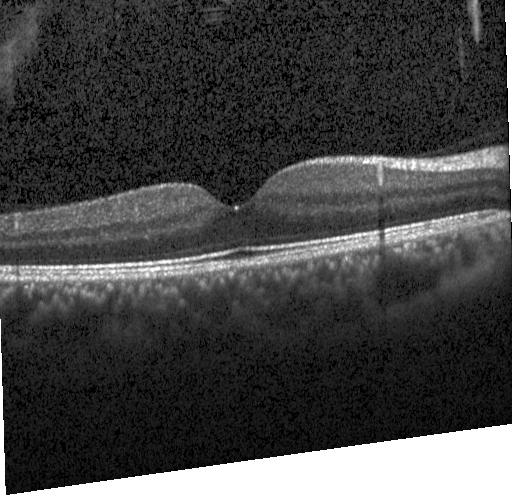

Optical coherence tomography B-scan. Heidelberg Spectralis. Fovea-centered. Spectral-domain OCT — Impression: no choroidal neovascularization, diabetic macular edema, or drusen.